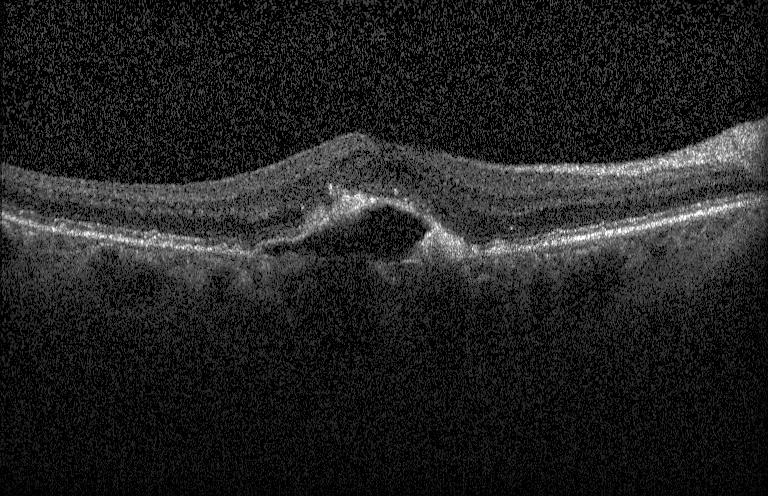
Retinal OCT B-scan, centered on the fovea.
Impression: CNV.